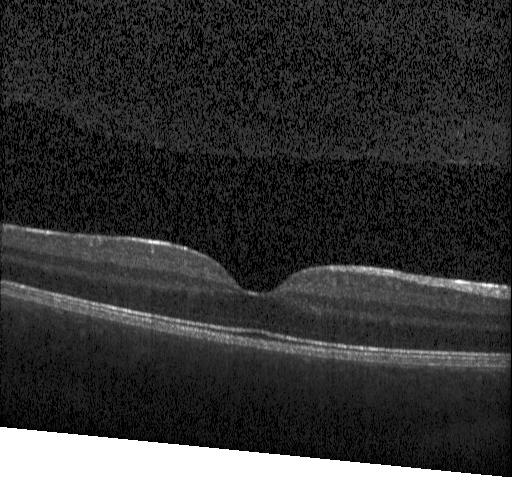
Retinal OCT cross-section showing no evidence of CNV, DME, or drusen.